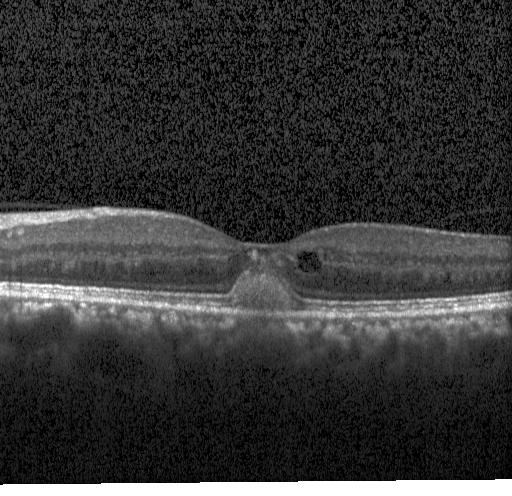 Impression: a choroidal neovascular membrane.